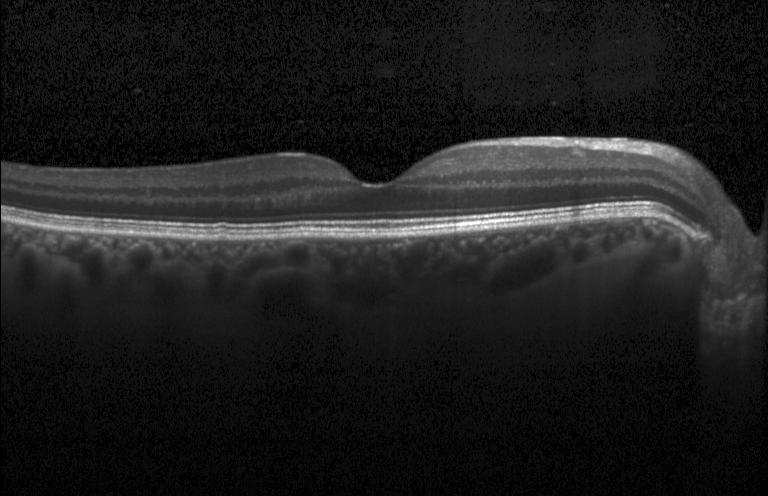

Optical coherence tomography B-scan — No CNV, no DME, and no drusen.